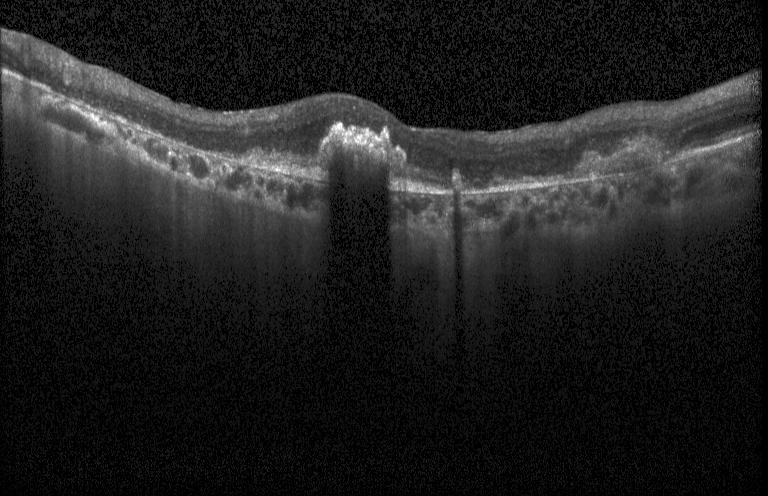 Heidelberg Spectralis · retinal OCT cross-section. The scan shows CNV.